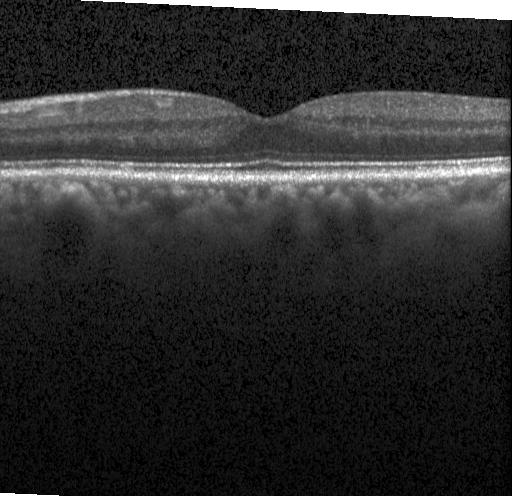
Through the macula, Heidelberg Spectralis, OCT B-scan
This B-scan demonstrates no choroidal neovascularization, diabetic macular edema, or drusen.